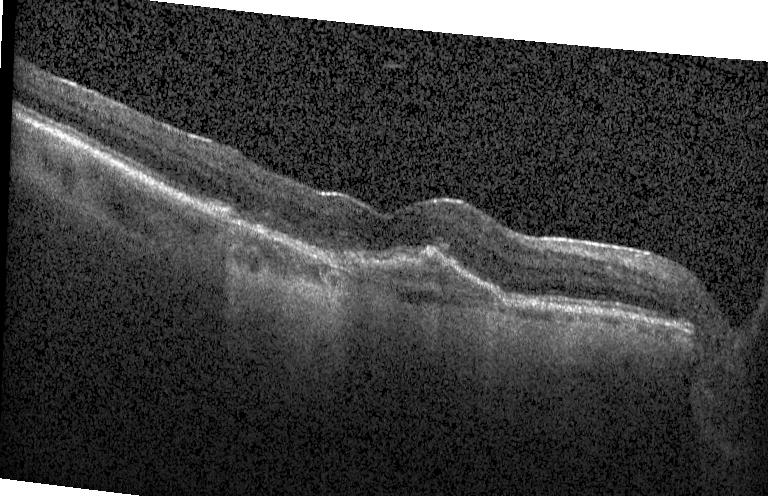 Spectral-domain OCT, Heidelberg Spectralis OCT system, horizontal scan through the fovea, OCT line scan. Finding: choroidal neovascularization (CNV).